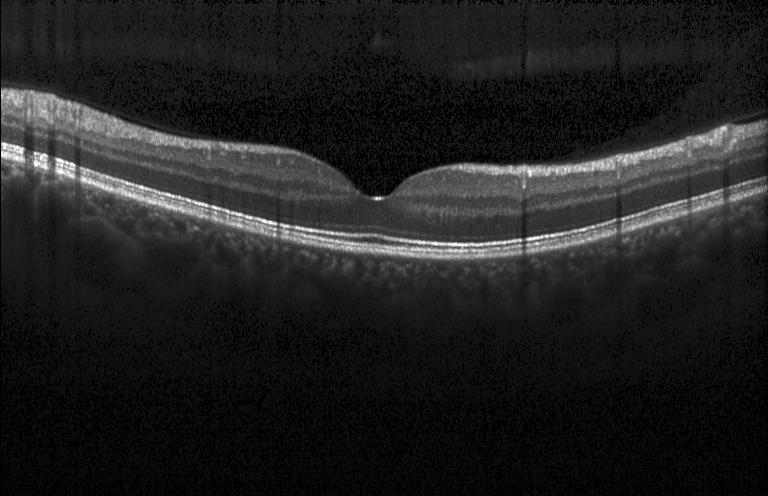

Through the macula; SD-OCT; Heidelberg Spectralis OCT system; optical coherence tomography B-scan — No choroidal neovascularization, diabetic macular edema, or drusen.